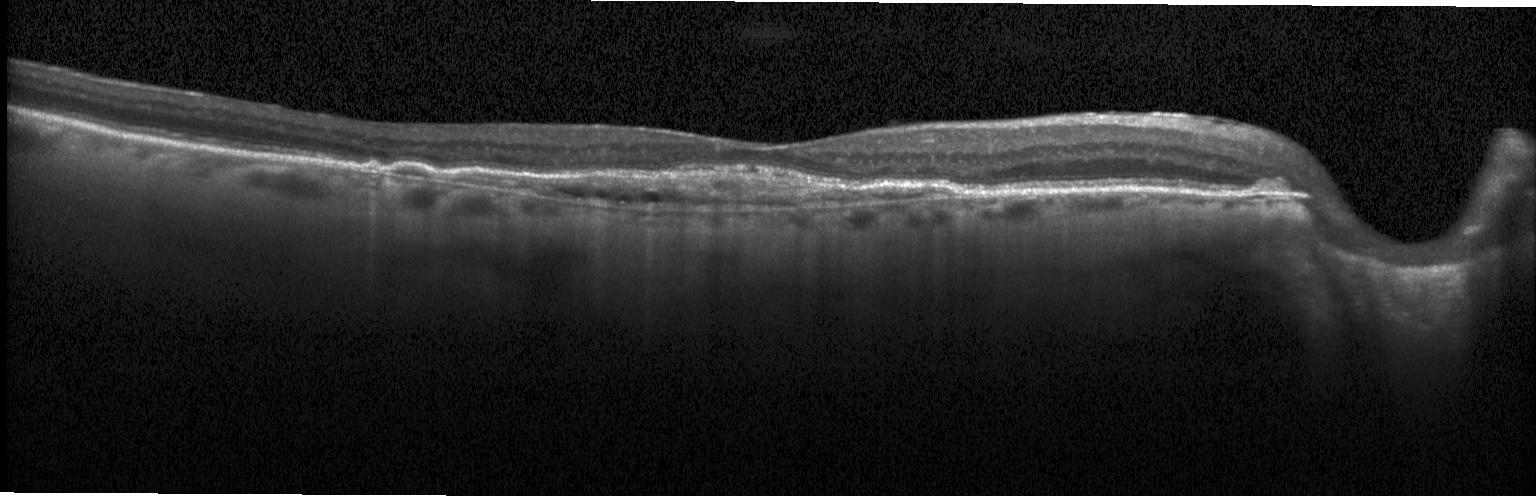
The scan shows choroidal neovascularization (CNV).